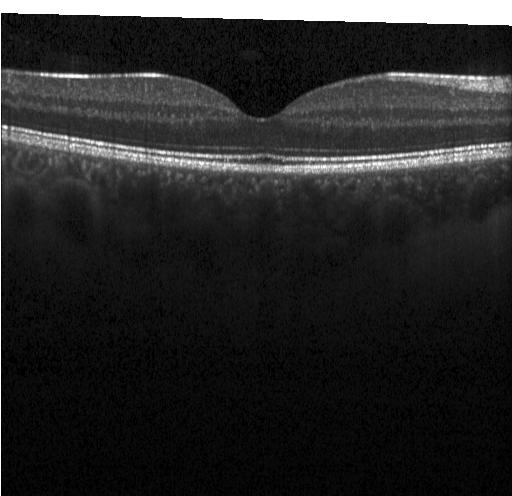
Optical coherence tomography scan · spectral-domain optical coherence tomography
This B-scan demonstrates no choroidal neovascularization, no diabetic macular edema, and no drusen.